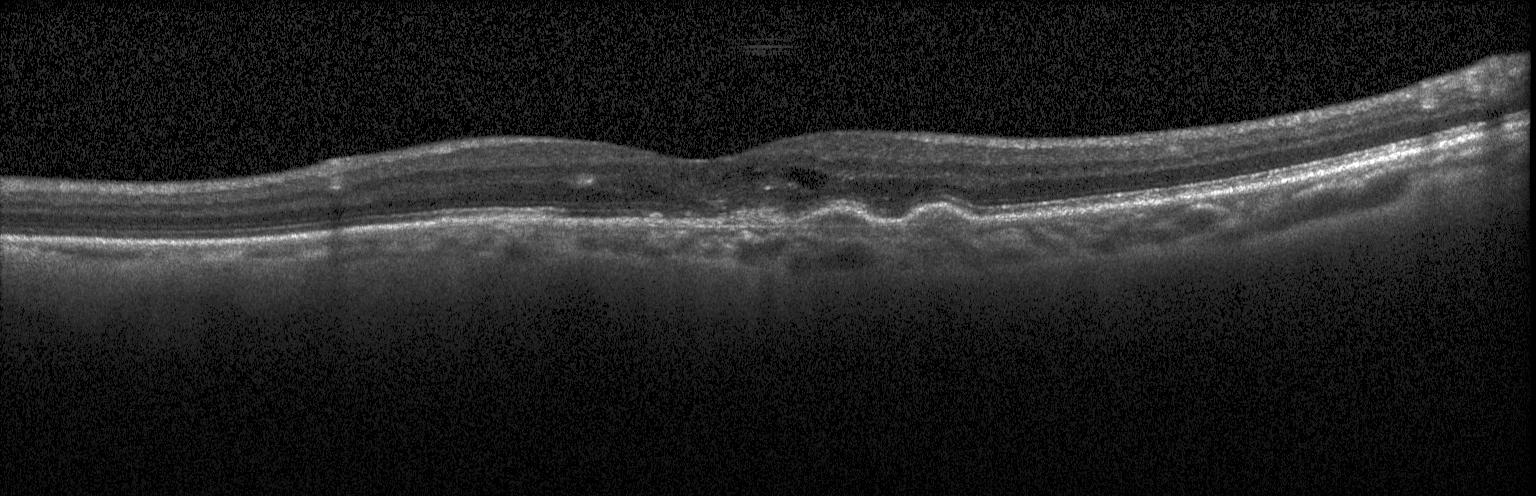

The scan shows a choroidal neovascular membrane.